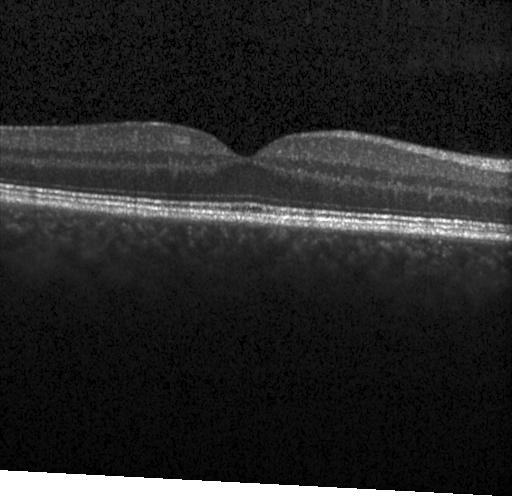
This B-scan demonstrates no choroidal neovascularization, diabetic macular edema, or drusen.